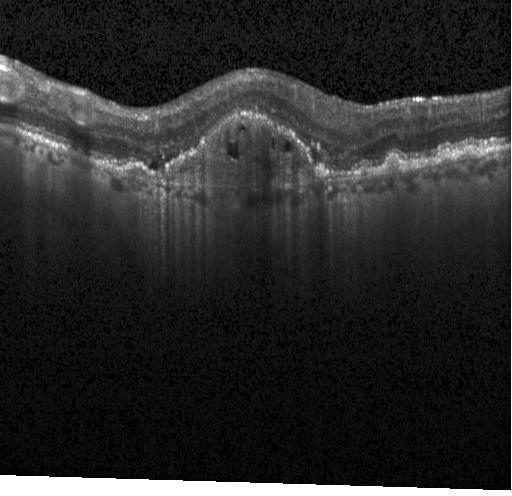
Spectral-domain OCT. Centered on the fovea. Retinal OCT cross-section.
This B-scan demonstrates a choroidal neovascular membrane.